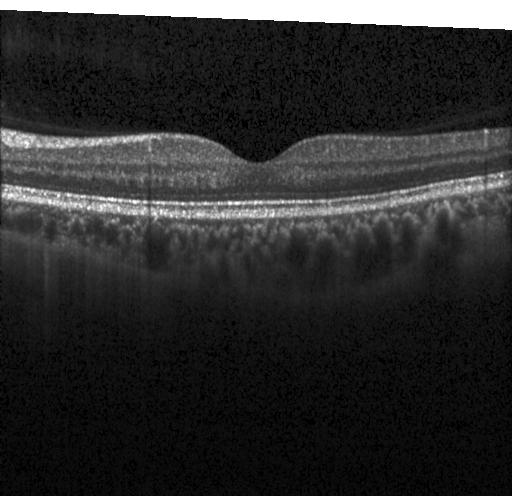

Horizontal scan through the fovea · retinal OCT cross-section — Finding: neither choroidal neovascularization, diabetic macular edema, nor drusen.